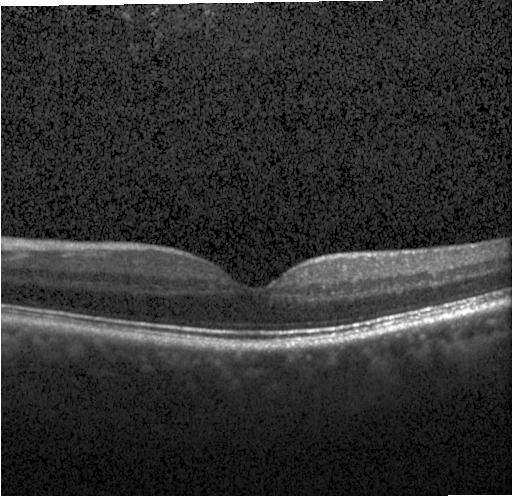
Optical coherence tomography scan, SD-OCT, centered on the fovea — The scan shows no CNV, no DME, and no drusen.